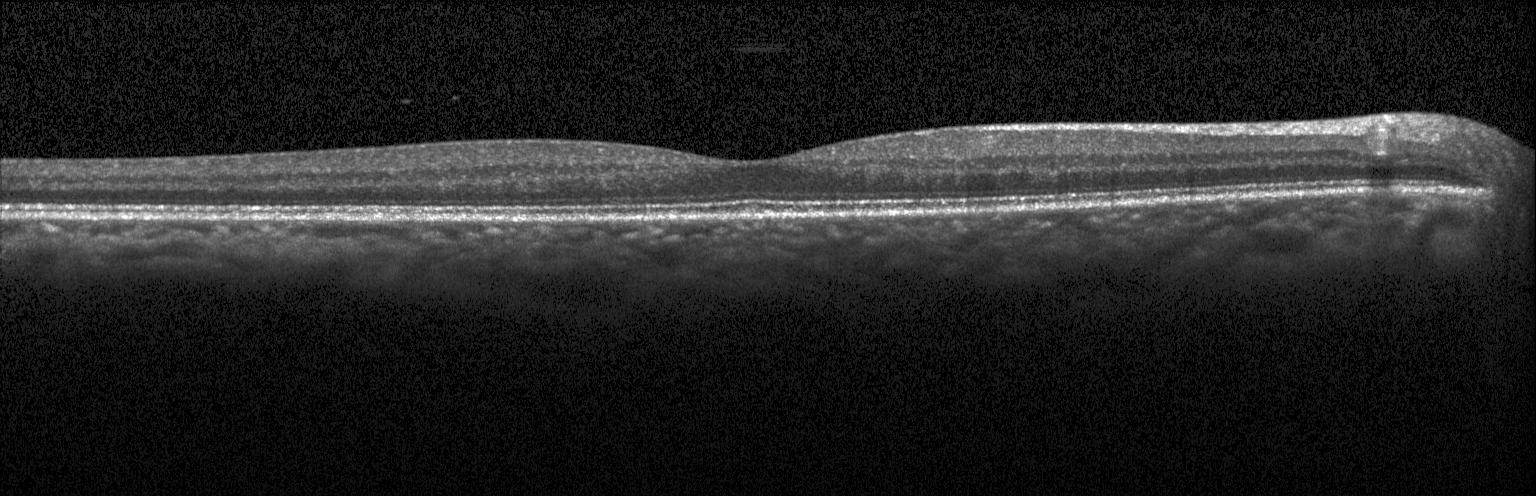

Macular scan, spectral-domain optical coherence tomography, instrument: Heidelberg Spectralis, OCT line scan. Neither choroidal neovascularization, diabetic macular edema, nor drusen.